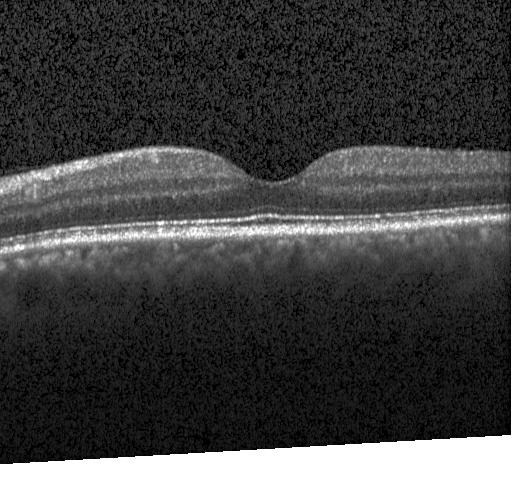 Instrument: Heidelberg Spectralis; spectral-domain optical coherence tomography; through the macula; retinal OCT cross-section
Diagnosis: no choroidal neovascularization, no diabetic macular edema, and no drusen.